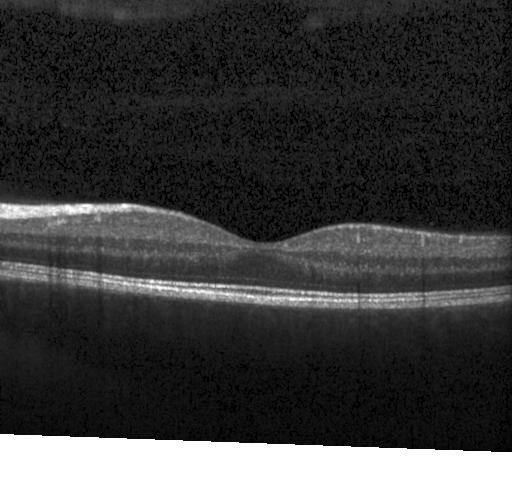 SD-OCT · optical coherence tomography B-scan.
Finding: neither choroidal neovascularization, diabetic macular edema, nor drusen.